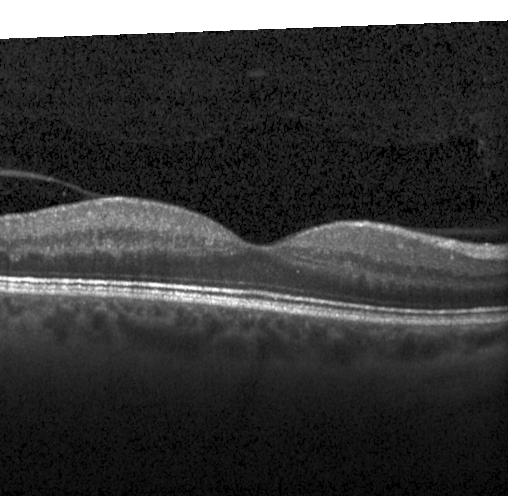 Retinal OCT cross-section; instrument: Heidelberg Spectralis. Assessment: no CNV, DME, or drusen.